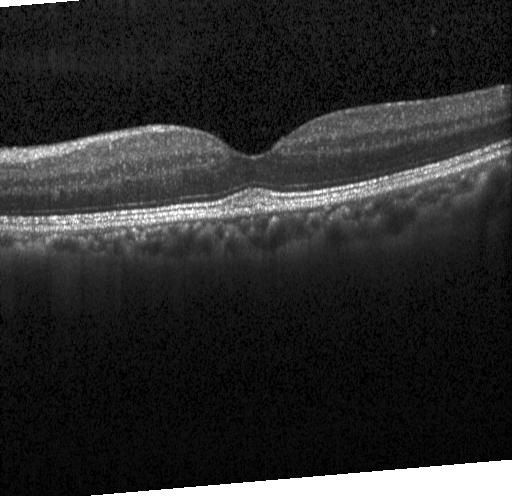 Macular scan; retinal OCT cross-section; Heidelberg Spectralis — Impression: no evidence of choroidal neovascularization, diabetic macular edema, or drusen.